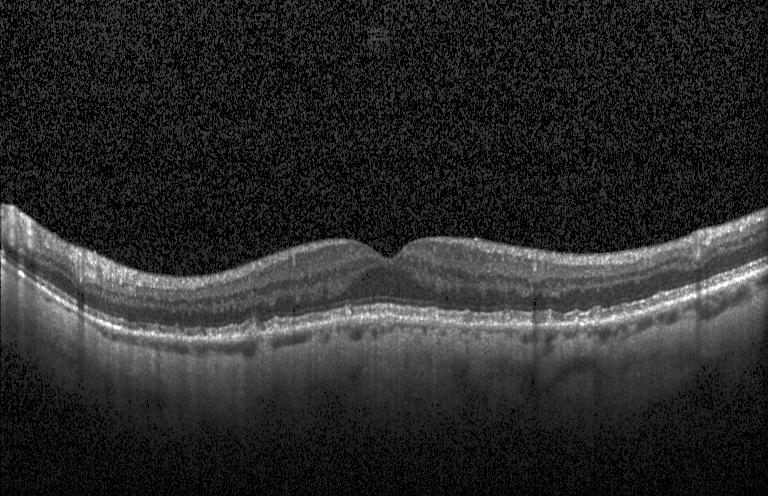
Macular OCT demonstrating multiple drusen.